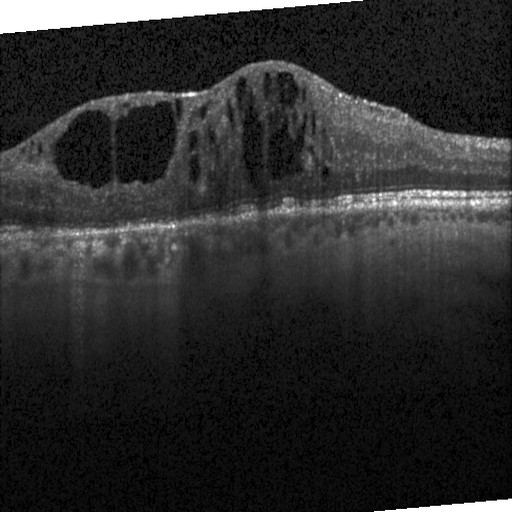

Fovea-centered; spectral-domain OCT; OCT B-scan; Heidelberg Spectralis
Assessment: diabetic macular edema (DME).